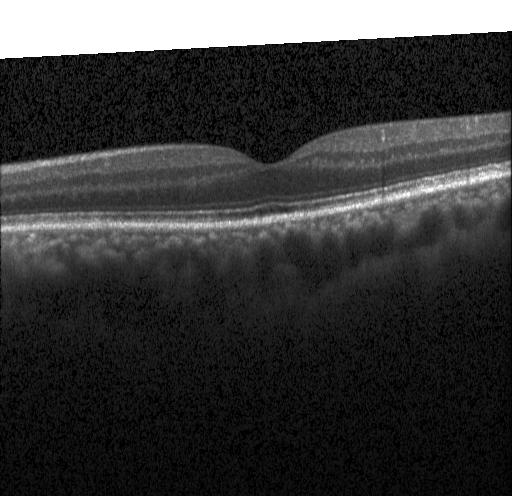

Centered on the fovea, OCT B-scan, spectral-domain optical coherence tomography.
Impression: no choroidal neovascularization, diabetic macular edema, or drusen.